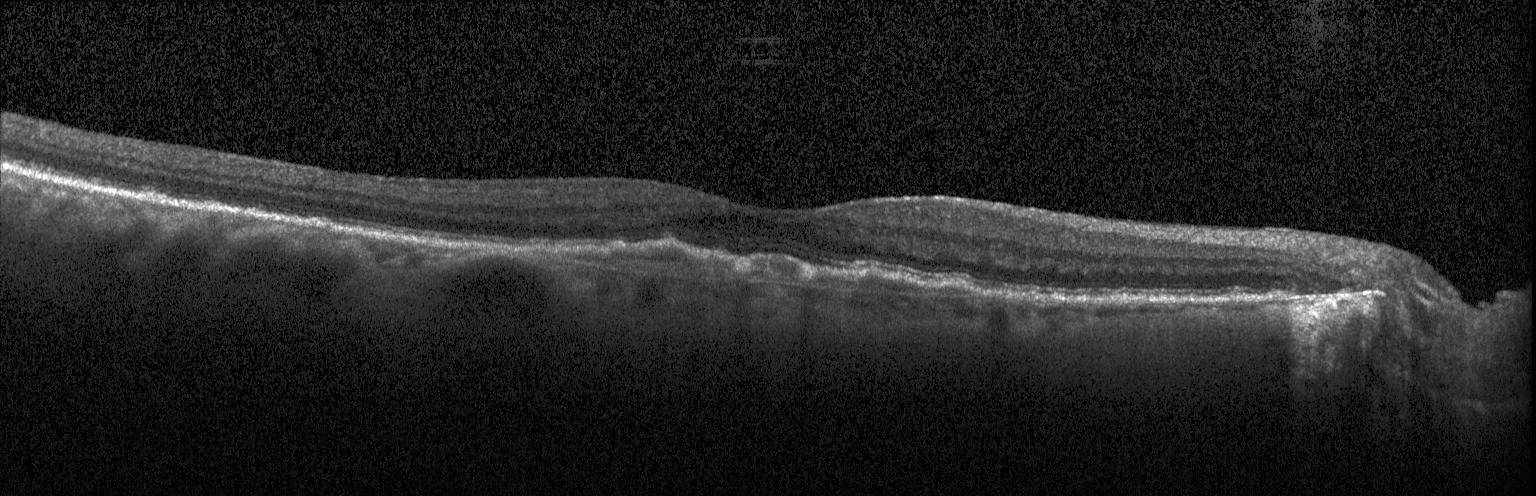 Heidelberg Spectralis; SD-OCT; centered on the fovea; optical coherence tomography scan
Assessment: choroidal neovascularization (CNV).